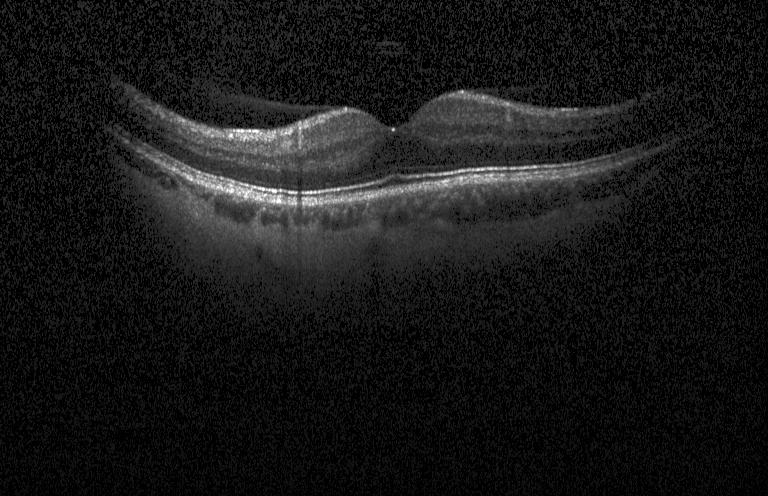 Assessment: no evidence of CNV, DME, or drusen.